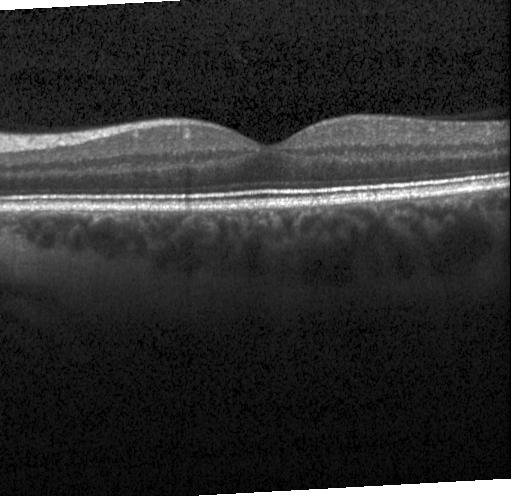 OCT line scan.
Neither choroidal neovascularization, diabetic macular edema, nor drusen.